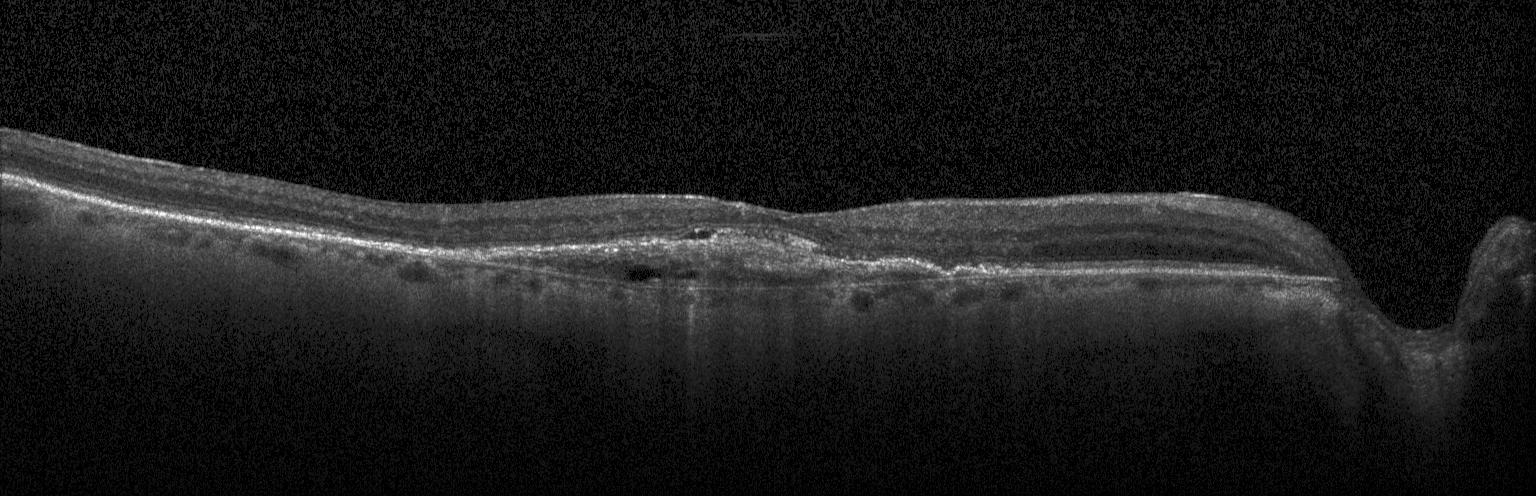 OCT B-scan · spectral-domain optical coherence tomography.
OCT finding: choroidal neovascularization.